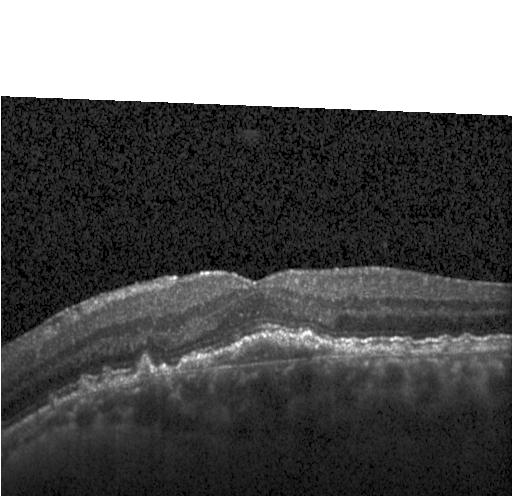 Impression: a choroidal neovascular membrane.